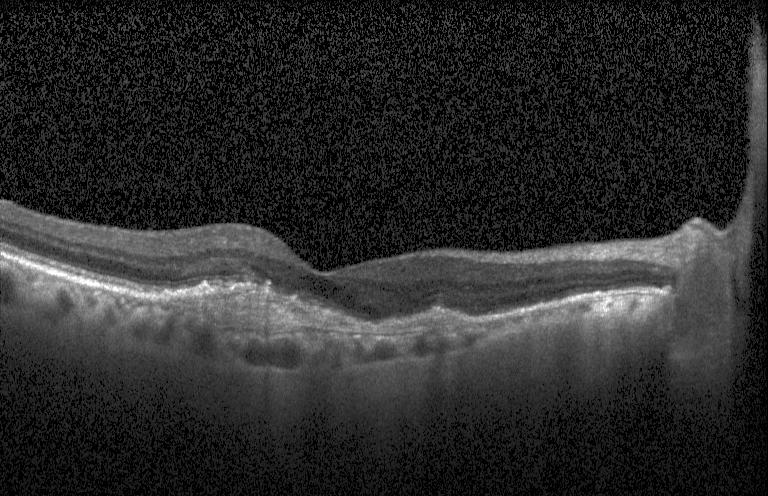 Retinal OCT cross-section. Fovea-centered. Instrument: Heidelberg Spectralis.
Impression: choroidal neovascularization.